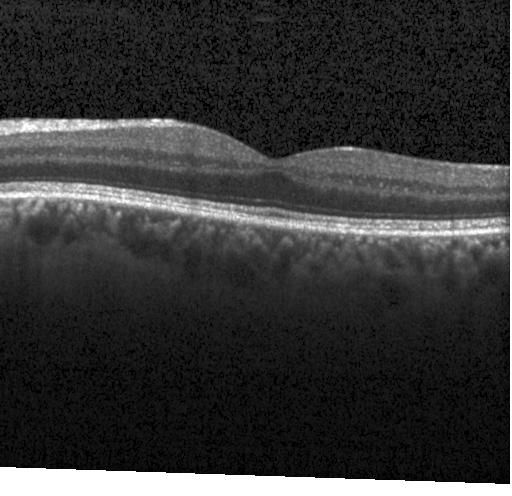

Diagnosis: no evidence of choroidal neovascularization, diabetic macular edema, or drusen.